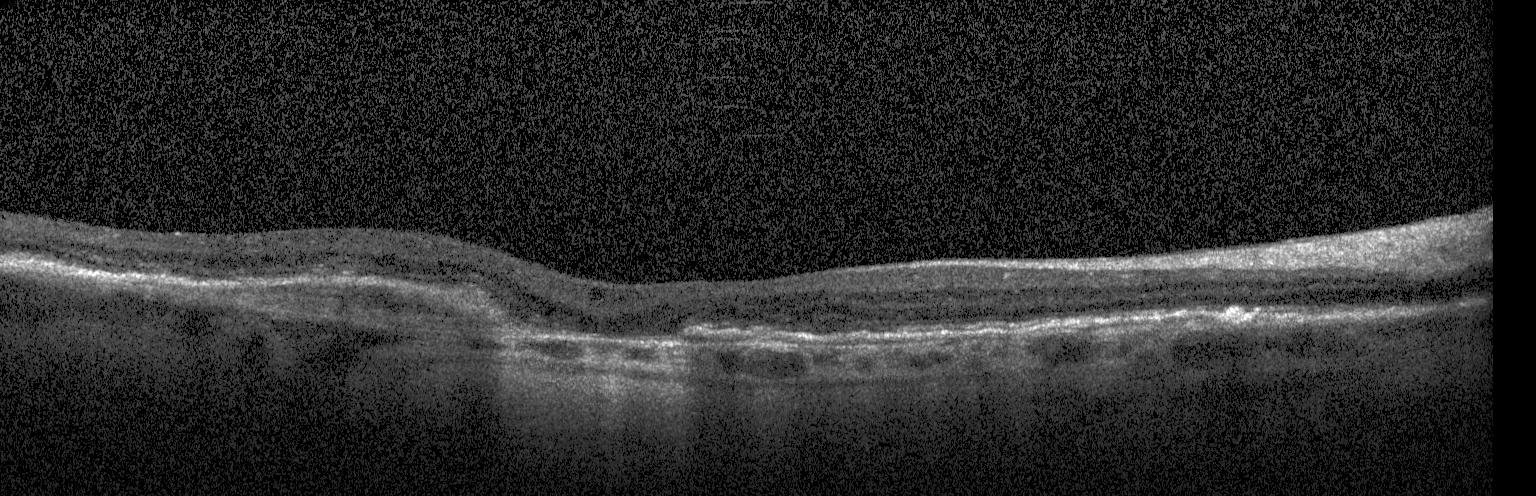

Retinal OCT cross-section, Heidelberg Spectralis OCT system, fovea-centered, SD-OCT. Finding: a choroidal neovascular membrane.